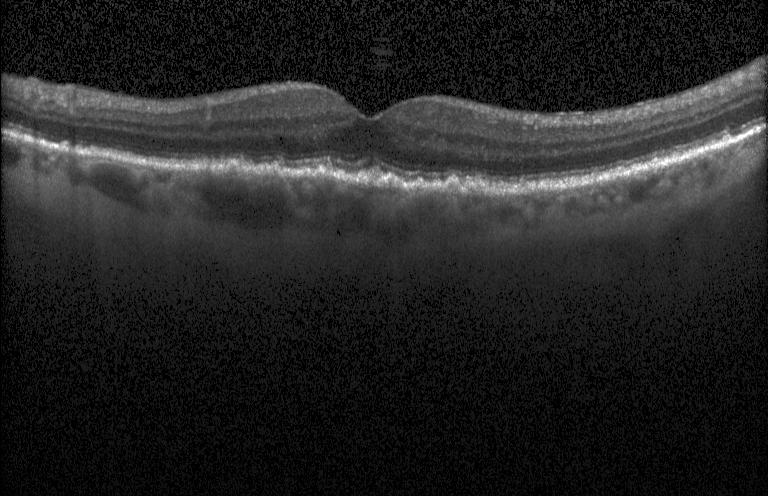
Impression: sub-RPE drusenoid deposits.